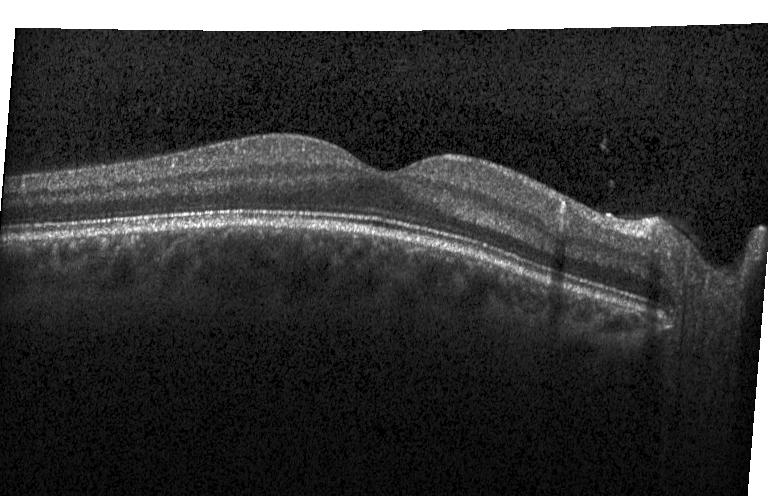

The scan shows no CNV, DME, or drusen.